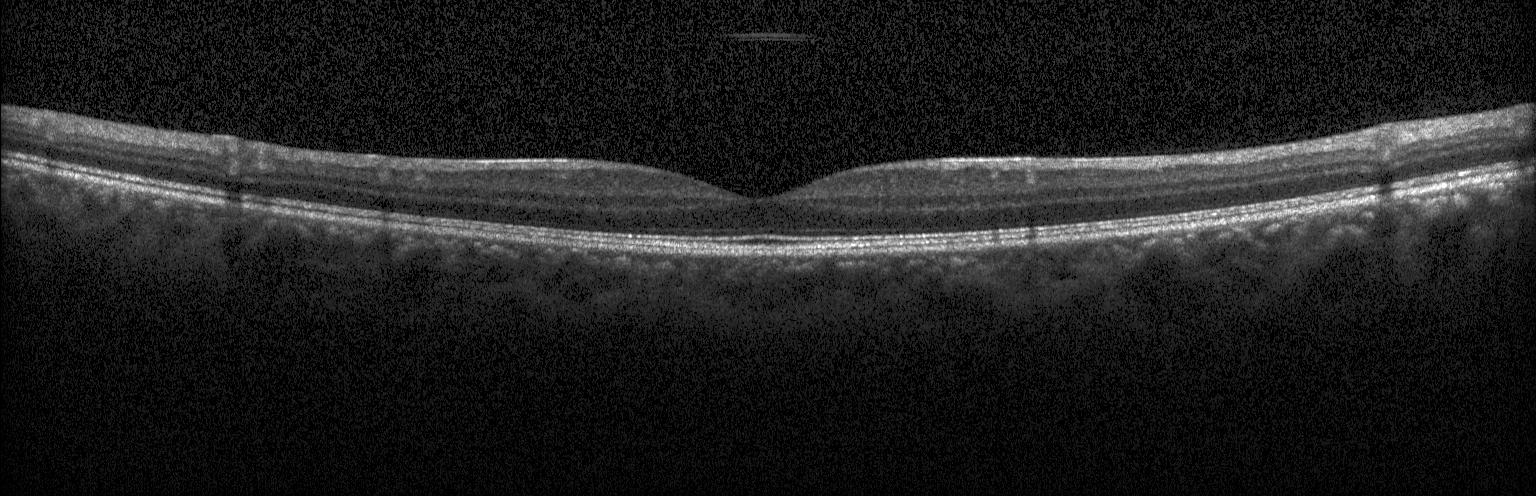
Heidelberg Spectralis, retinal OCT B-scan, spectral-domain optical coherence tomography — This B-scan demonstrates no evidence of choroidal neovascularization, diabetic macular edema, or drusen.